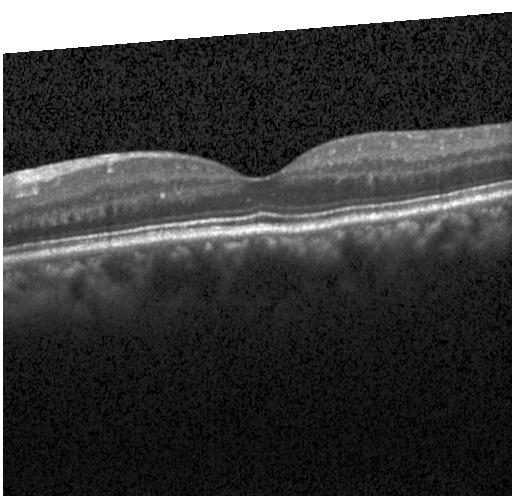 Heidelberg Spectralis OCT system, horizontal scan through the fovea, OCT B-scan. Diagnosis: neither CNV, DME, nor drusen.